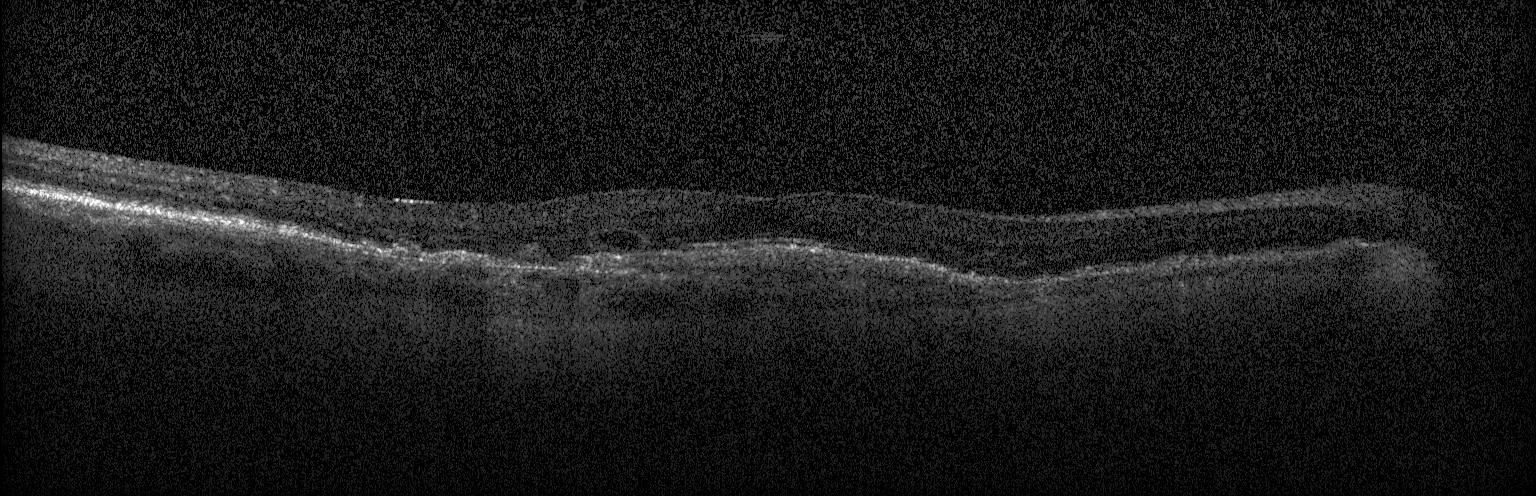 OCT B-scan · centered on the fovea · spectral-domain OCT · instrument: Heidelberg Spectralis
Diagnosis: choroidal neovascularization (CNV).